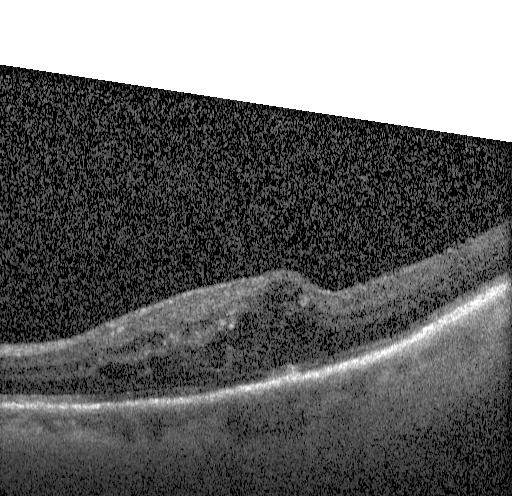

Optical coherence tomography scan. Diabetic macular edema.